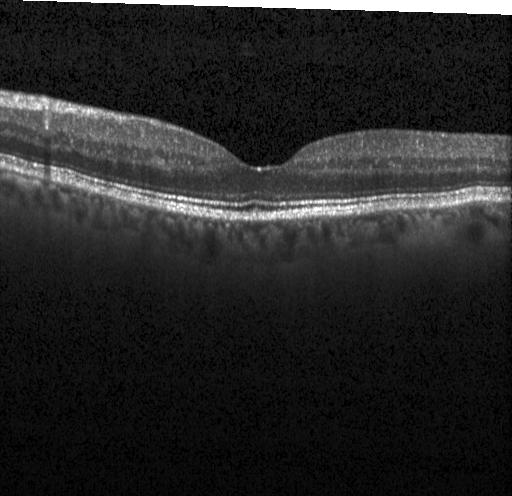
Optical coherence tomography scan — No evidence of choroidal neovascularization, diabetic macular edema, or drusen.